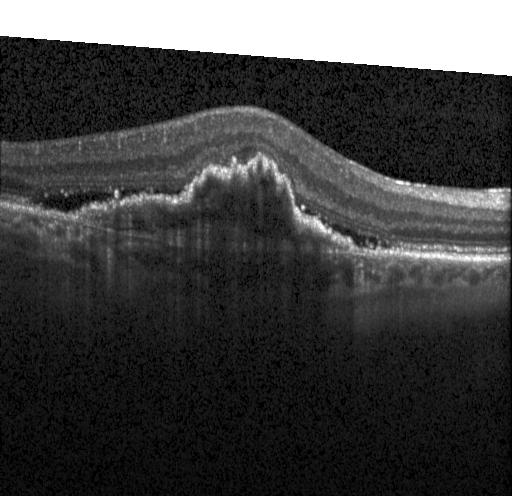

Diagnosis: a choroidal neovascular membrane.